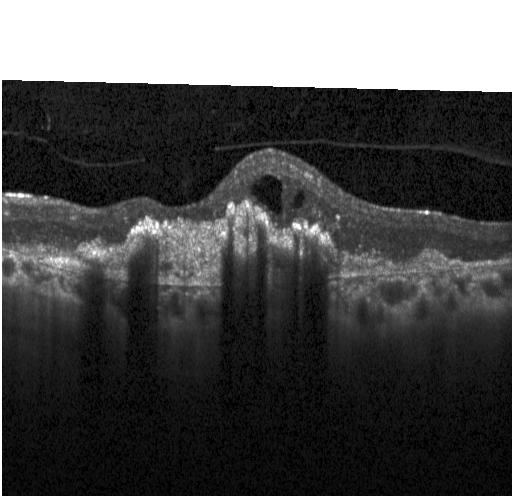

Optical coherence tomography scan. Impression: choroidal neovascularization (CNV).